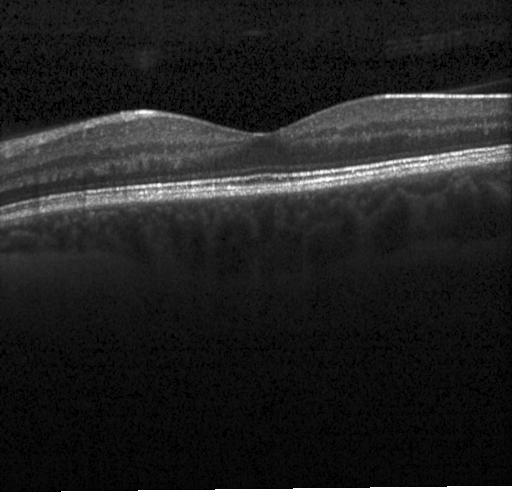
Spectral-domain OCT; horizontal scan through the fovea; Heidelberg Spectralis OCT system; retinal OCT cross-section. Macular OCT: no CNV, DME, or drusen.